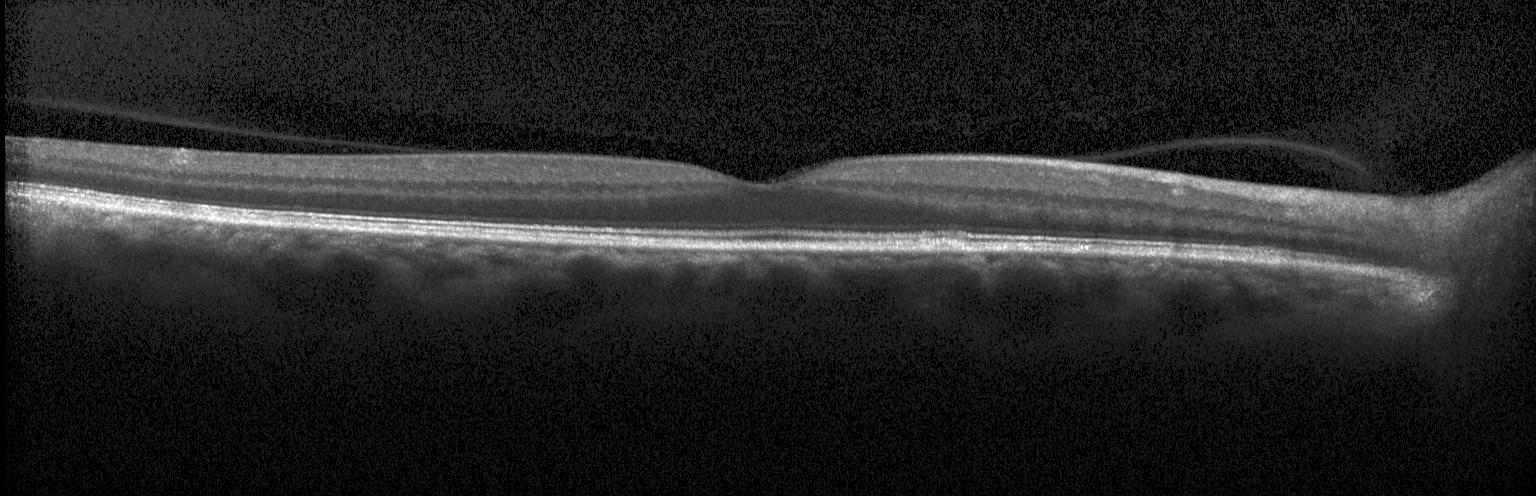

Finding: no choroidal neovascularization, no diabetic macular edema, and no drusen.